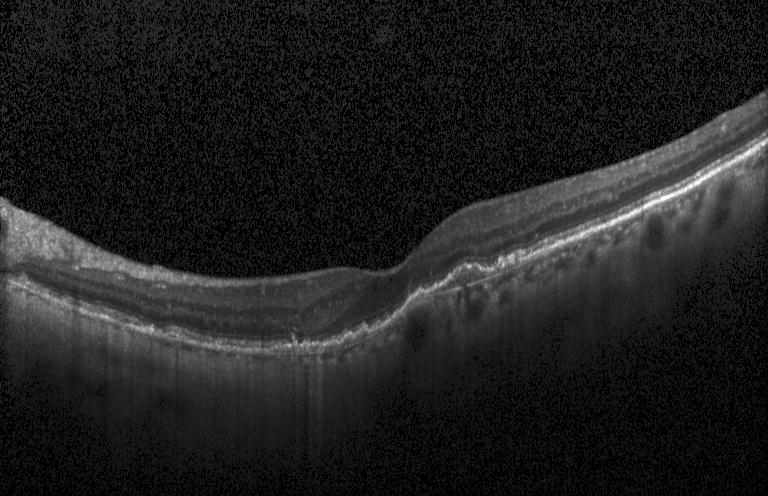 Heidelberg Spectralis; fovea-centered; OCT line scan — Assessment: choroidal neovascularization.